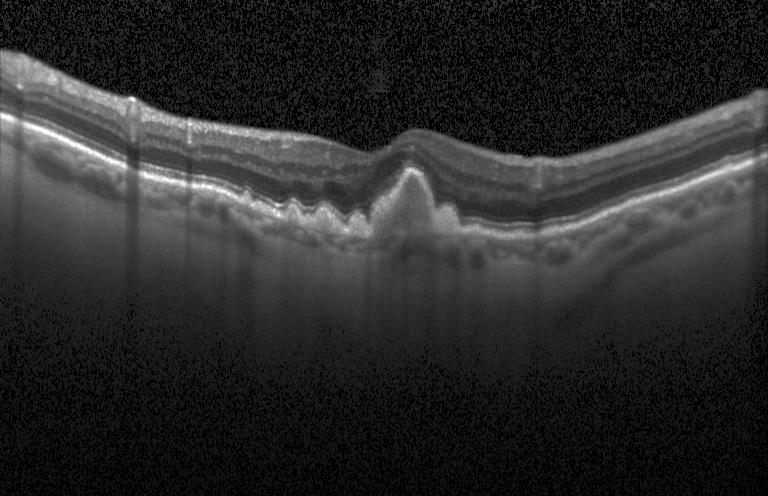

OCT B-scan
This B-scan demonstrates sub-RPE drusenoid deposits.